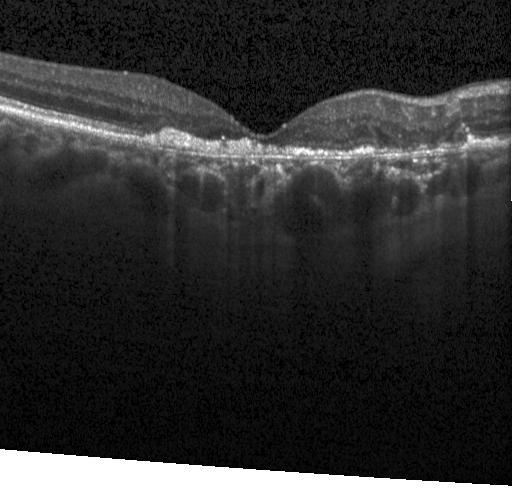

Finding: choroidal neovascularization (CNV).